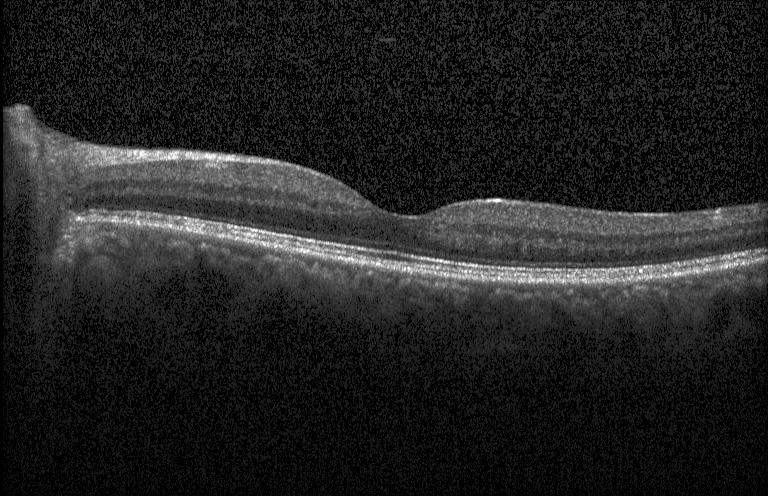

Acquired on a Heidelberg Spectralis, OCT B-scan, fovea-centered
Impression: neither choroidal neovascularization, diabetic macular edema, nor drusen.